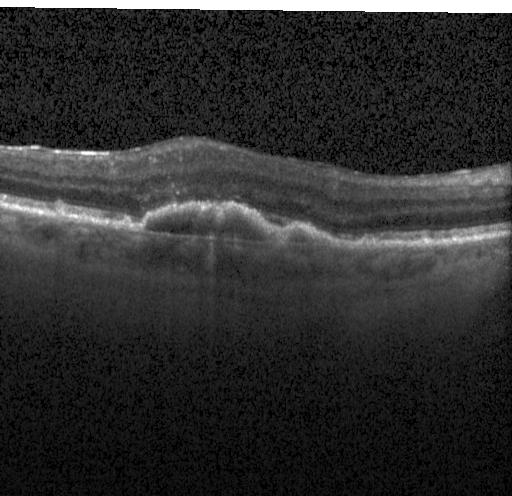

Optical coherence tomography scan. Diagnosis: a choroidal neovascular membrane.